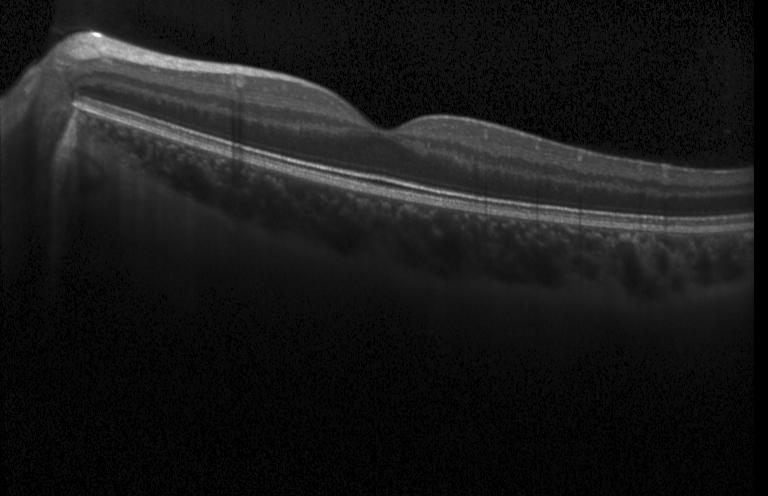 Retinal OCT cross-section — This B-scan demonstrates no CNV, no DME, and no drusen.